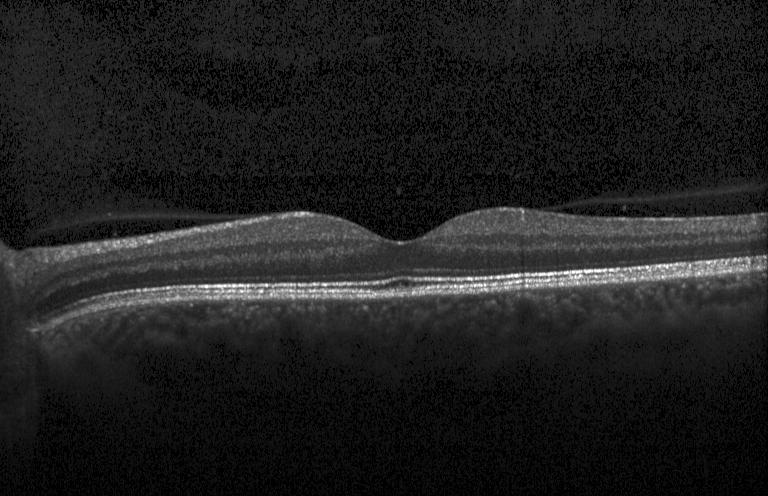

Instrument: Heidelberg Spectralis, fovea-centered, retinal OCT B-scan. No CNV, DME, or drusen.